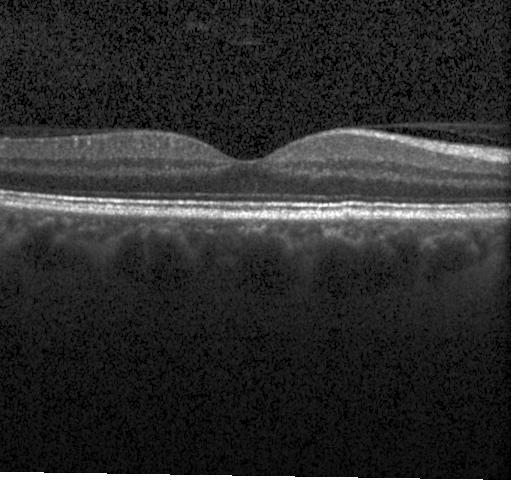

Optical coherence tomography scan. Neither CNV, DME, nor drusen.